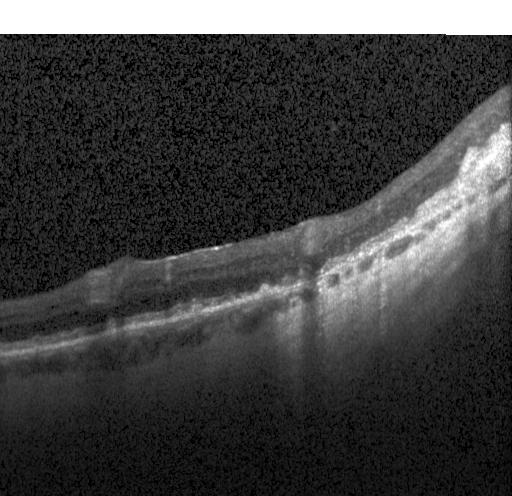
Optical coherence tomography scan — Dx: CNV.